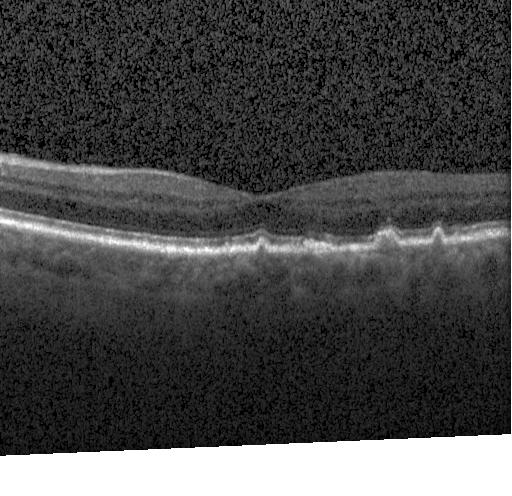

Macular scan; acquired on a Heidelberg Spectralis; SD-OCT; OCT B-scan
Finding: sub-RPE drusenoid deposits.